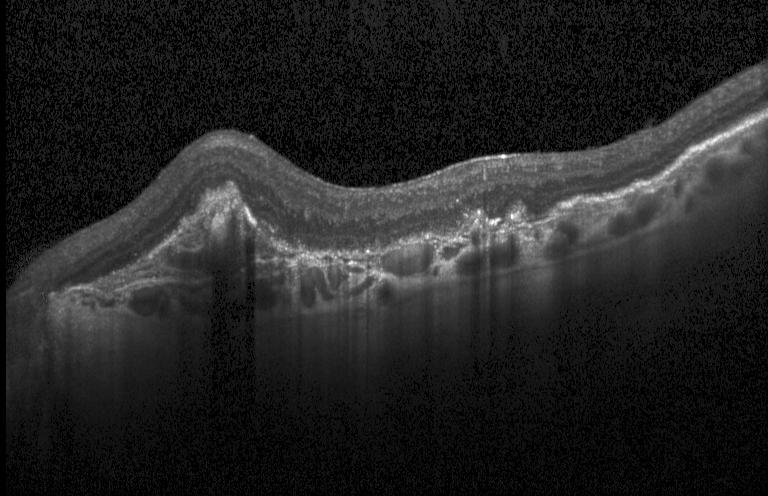

OCT scan showing choroidal neovascularization (CNV).